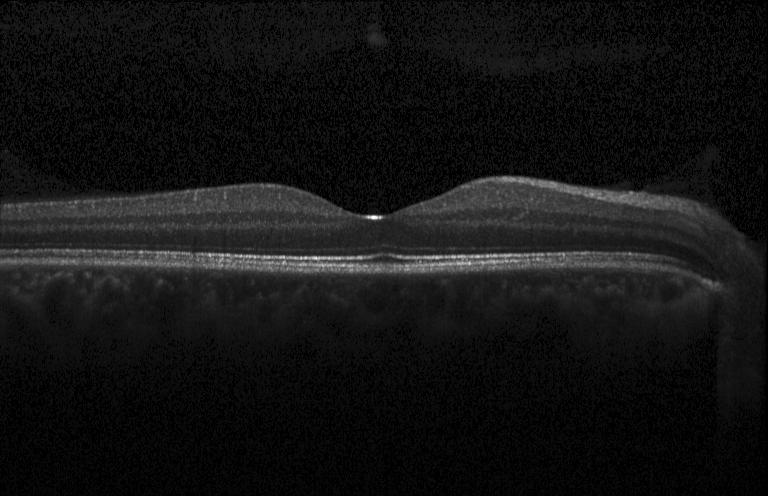
Optical coherence tomography scan
Macular OCT: neither CNV, DME, nor drusen.